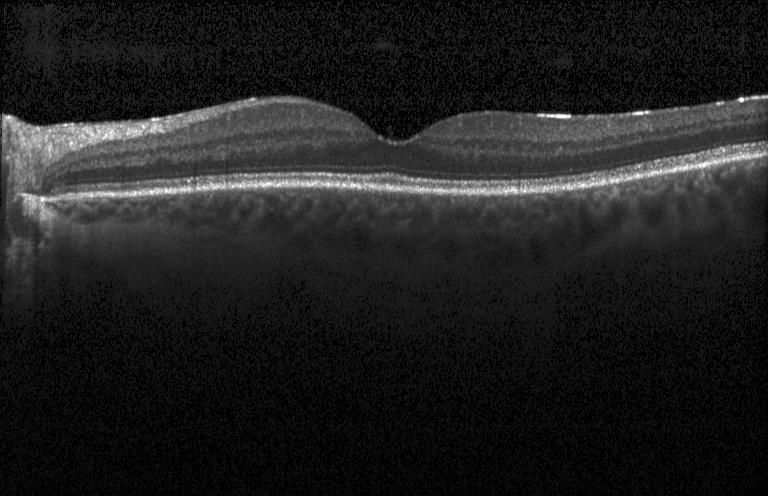
Centered on the fovea, OCT line scan
The scan shows no choroidal neovascularization, diabetic macular edema, or drusen.